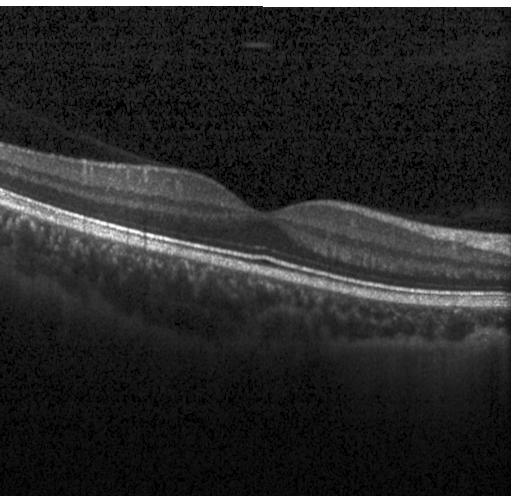 OCT finding: no choroidal neovascularization, diabetic macular edema, or drusen.